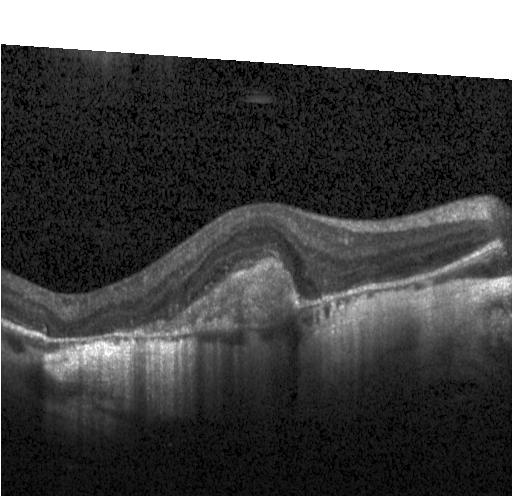

This B-scan demonstrates a choroidal neovascular membrane.